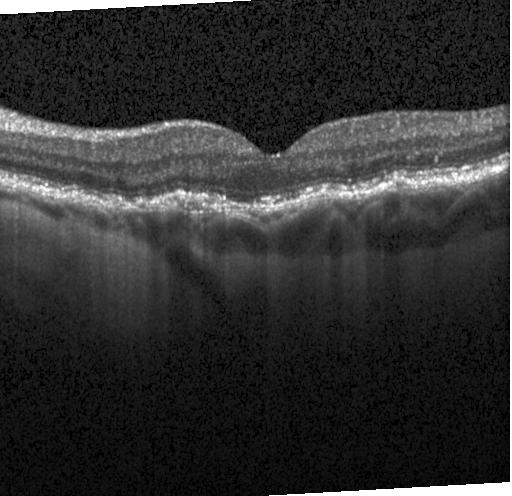 OCT line scan
Assessment: a choroidal neovascular membrane.